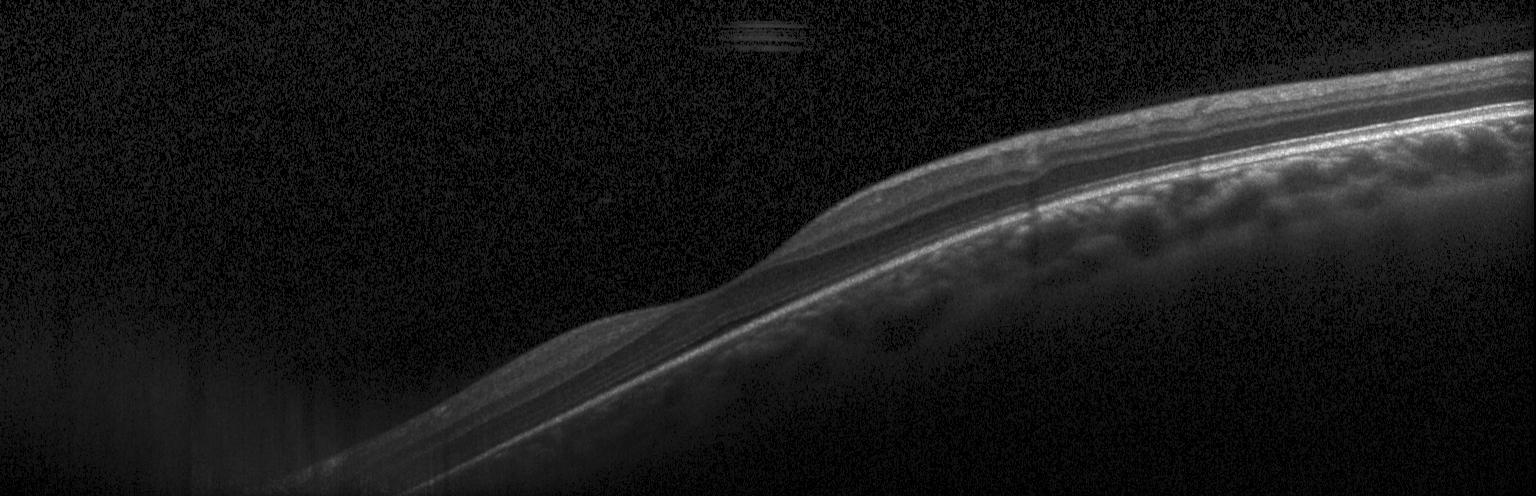 Optical coherence tomography scan.
Dx: no evidence of choroidal neovascularization, diabetic macular edema, or drusen.